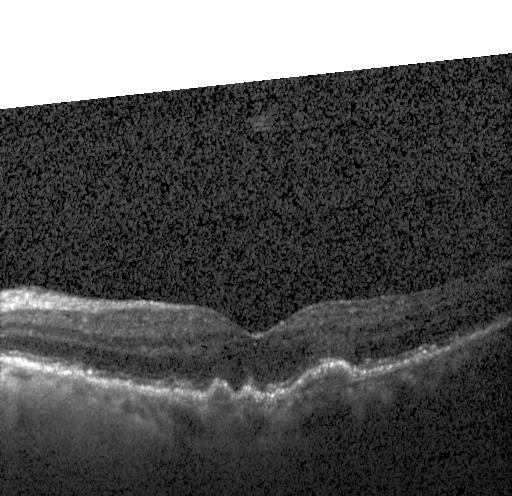 Spectral-domain OCT; optical coherence tomography scan; instrument: Heidelberg Spectralis.
Diagnosis: a choroidal neovascular membrane.